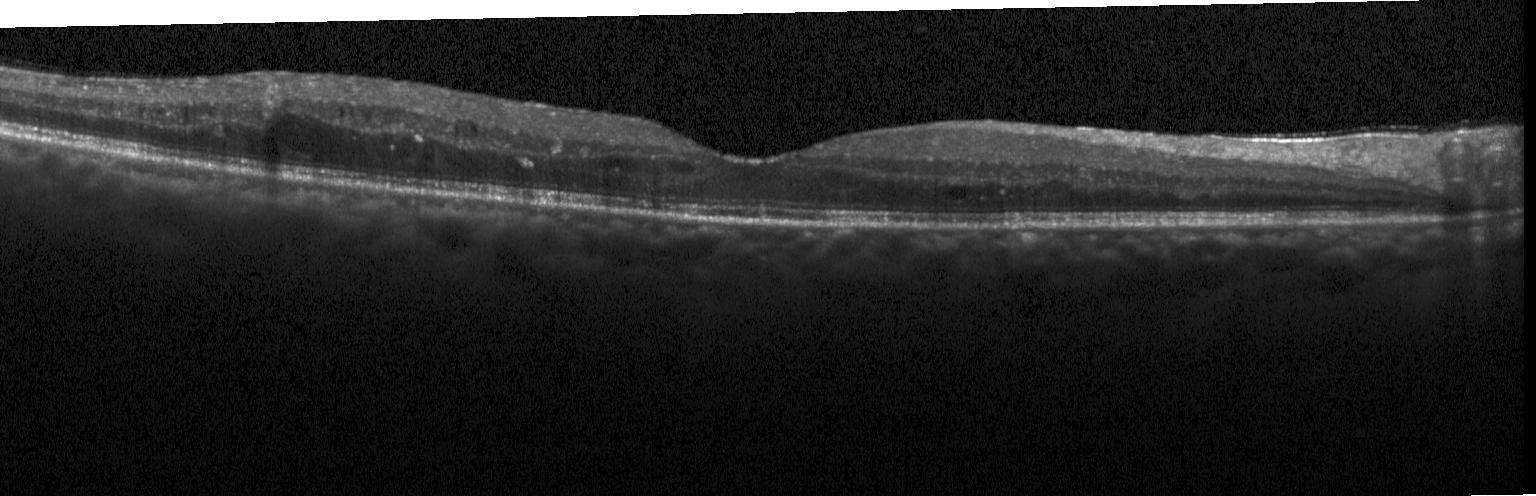
Heidelberg Spectralis, horizontal scan through the fovea, spectral-domain optical coherence tomography, optical coherence tomography scan.
The scan shows diabetic macular edema (DME).